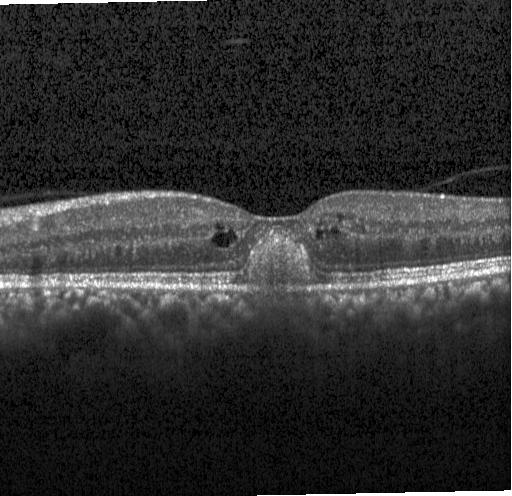
Dx: a choroidal neovascular membrane.